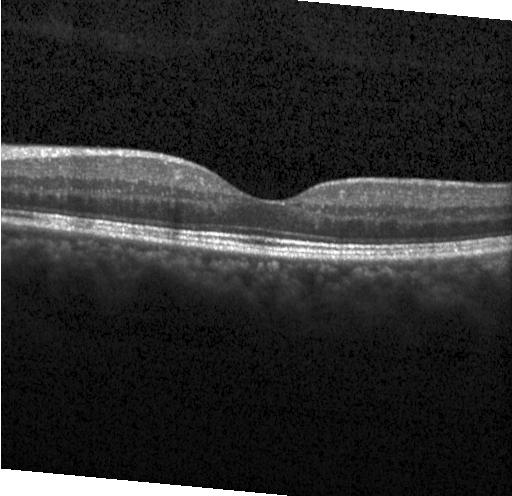

Spectral-domain OCT · macular scan · optical coherence tomography B-scan. OCT finding: no CNV, DME, or drusen.